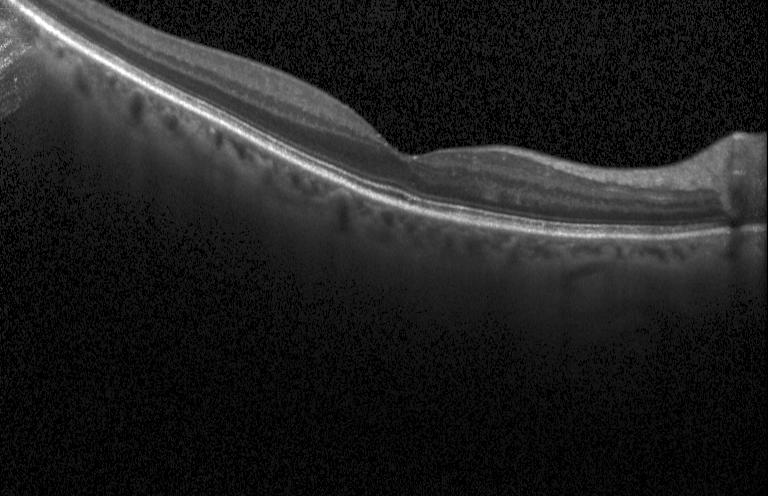 SD-OCT; OCT B-scan
Impression: neither CNV, DME, nor drusen.